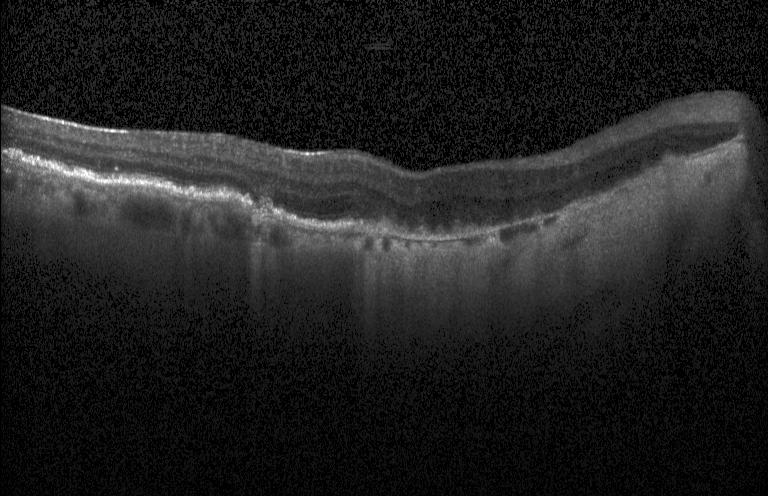

Spectral-domain OCT B-scan: a choroidal neovascular membrane.